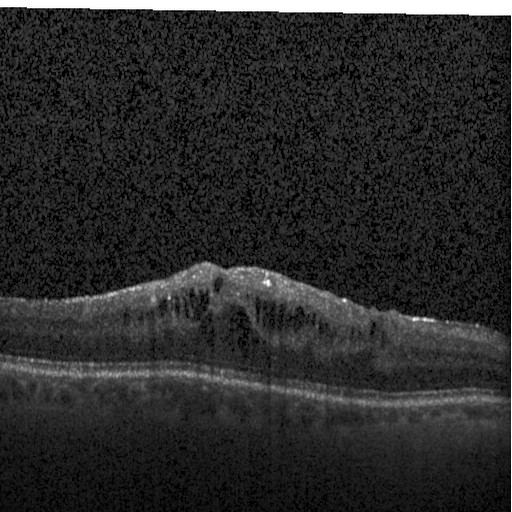
Macular OCT: DME.